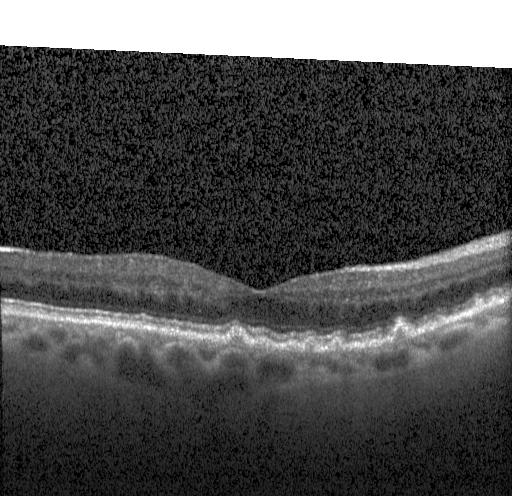
The scan shows sub-RPE drusenoid deposits.